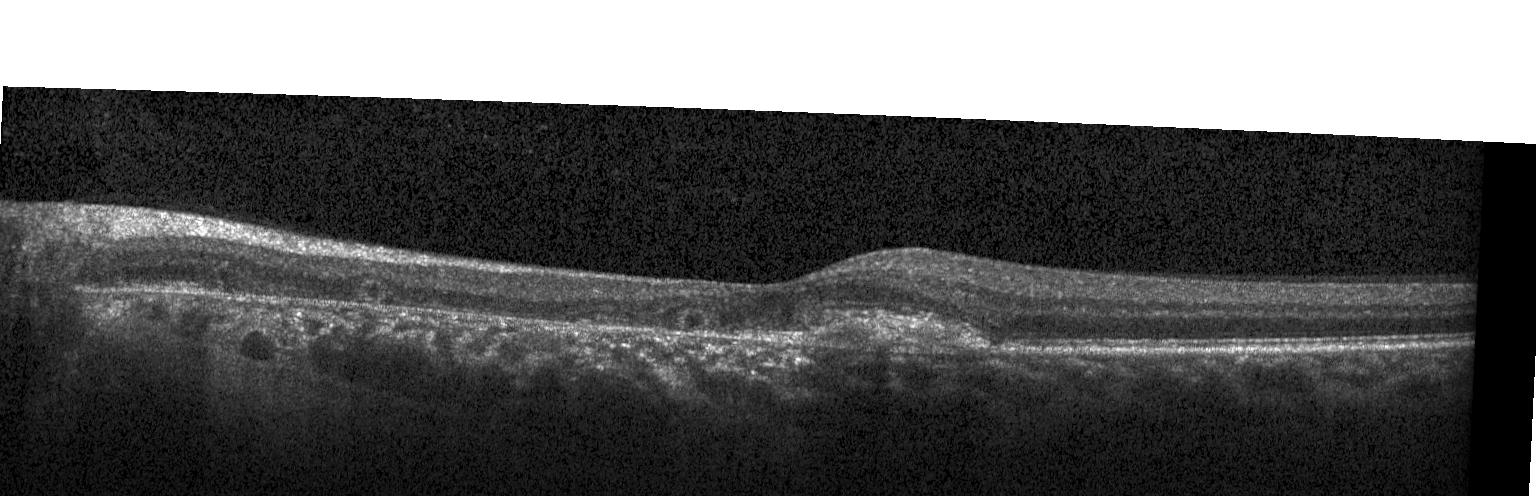

Optical coherence tomography scan; spectral-domain OCT — The scan shows a choroidal neovascular membrane.